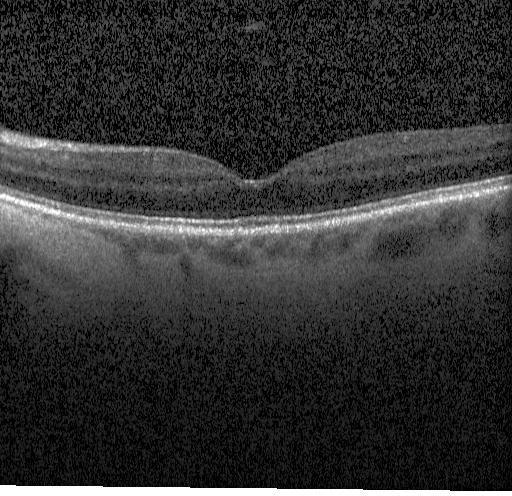

OCT B-scan. SD-OCT. Heidelberg Spectralis. Fovea-centered
This B-scan demonstrates neither choroidal neovascularization, diabetic macular edema, nor drusen.